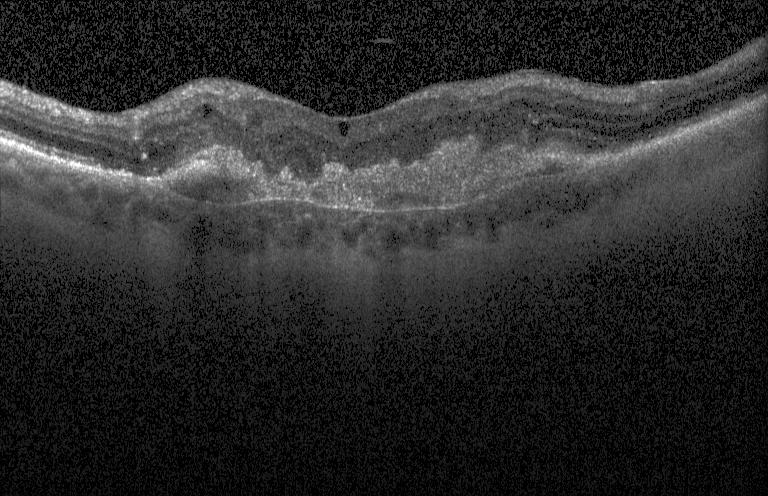 Macular scan · retinal OCT B-scan — Macular OCT: choroidal neovascularization.